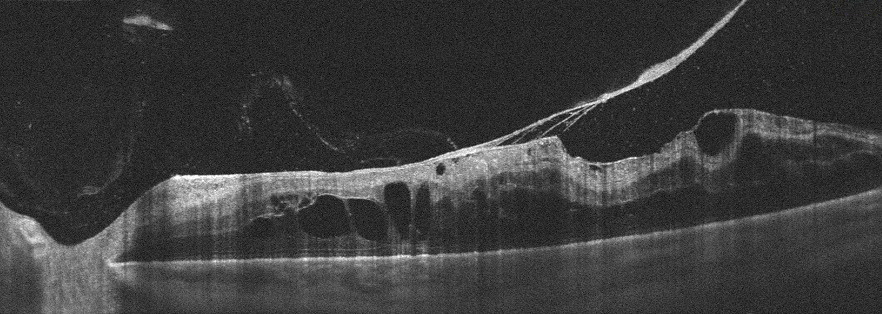 OCT scan showing DME.